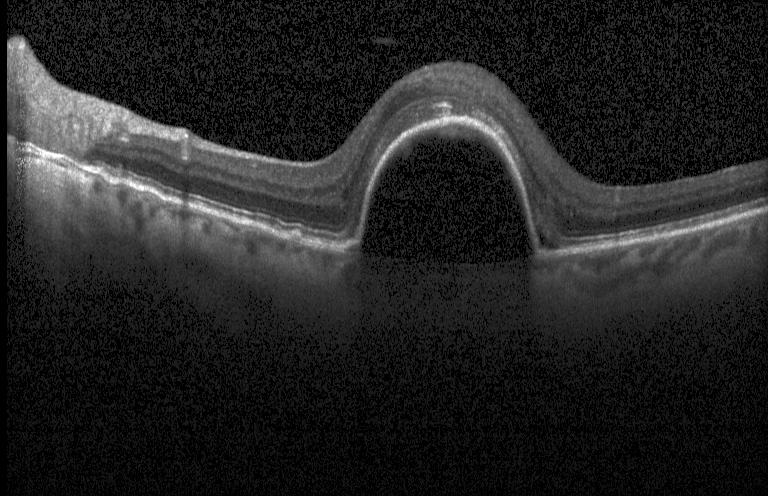
Horizontal scan through the fovea. OCT line scan. Heidelberg Spectralis OCT system. Spectral-domain OCT. Impression: a choroidal neovascular membrane.